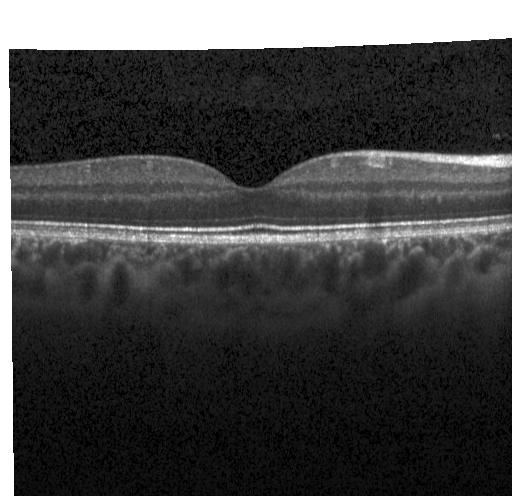

Horizontal scan through the fovea. Optical coherence tomography B-scan. Spectral-domain optical coherence tomography — Macular OCT: no choroidal neovascularization, no diabetic macular edema, and no drusen.